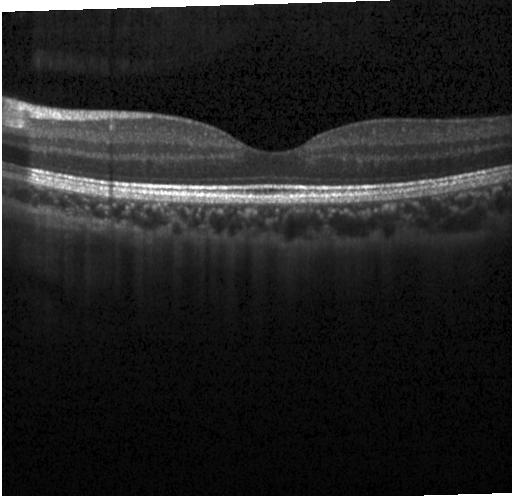

OCT B-scan
Dx: no CNV, DME, or drusen.